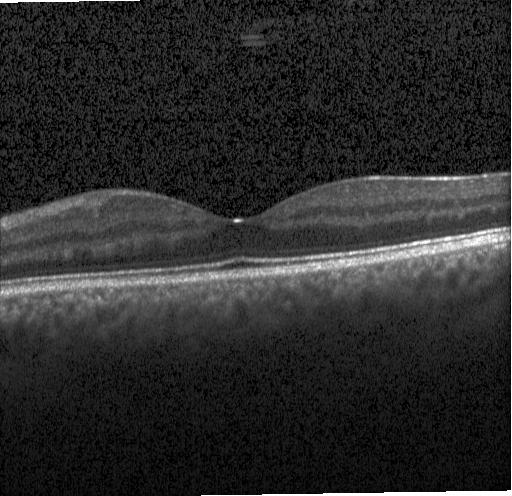
Centered on the fovea; instrument: Heidelberg Spectralis; optical coherence tomography B-scan.
Diagnosis: no choroidal neovascularization, no diabetic macular edema, and no drusen.